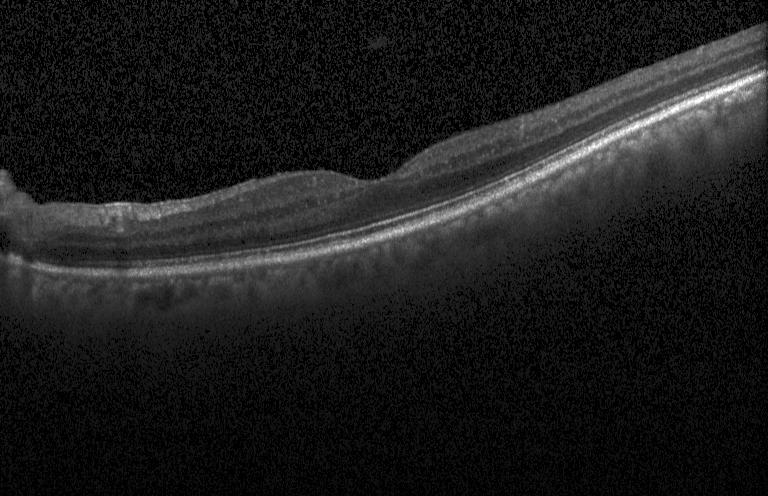 SD-OCT · optical coherence tomography scan. Finding: no CNV, no DME, and no drusen.